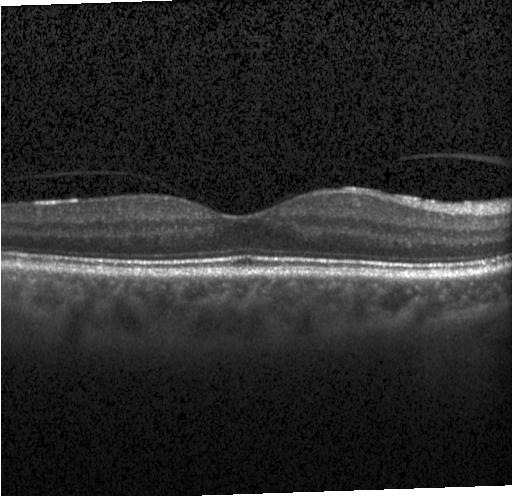

Retinal OCT B-scan. Assessment: no CNV, no DME, and no drusen.